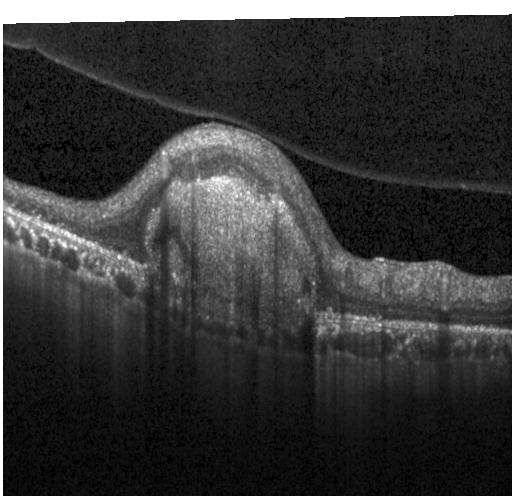
Diagnosis: choroidal neovascularization.